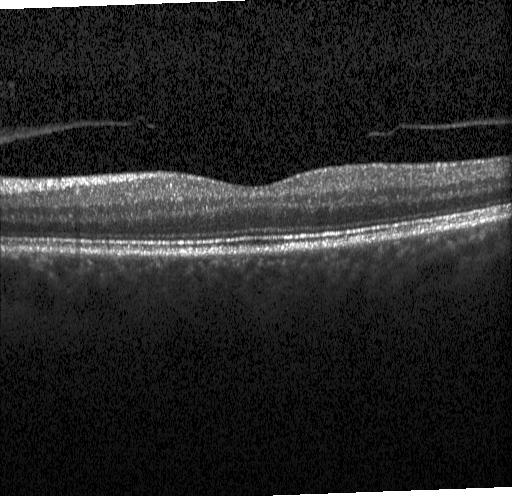

Retinal OCT B-scan — The scan shows no evidence of CNV, DME, or drusen.